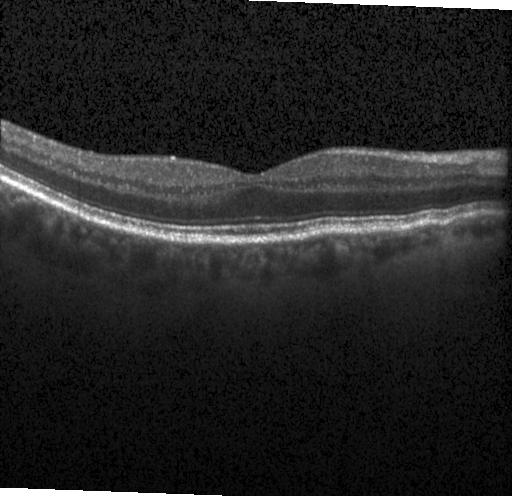 OCT B-scan showing no CNV, DME, or drusen.